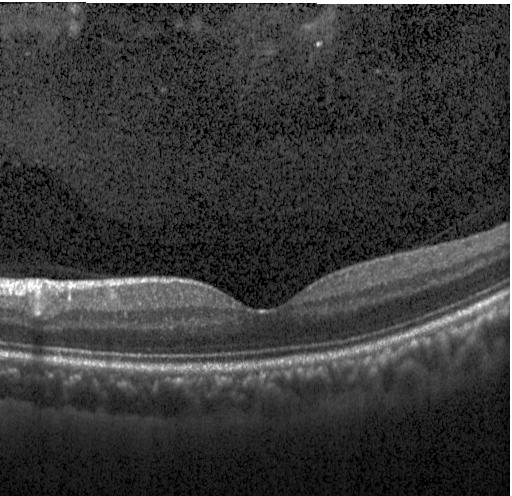

Retinal OCT cross-section; centered on the fovea — Diagnosis: no evidence of CNV, DME, or drusen.